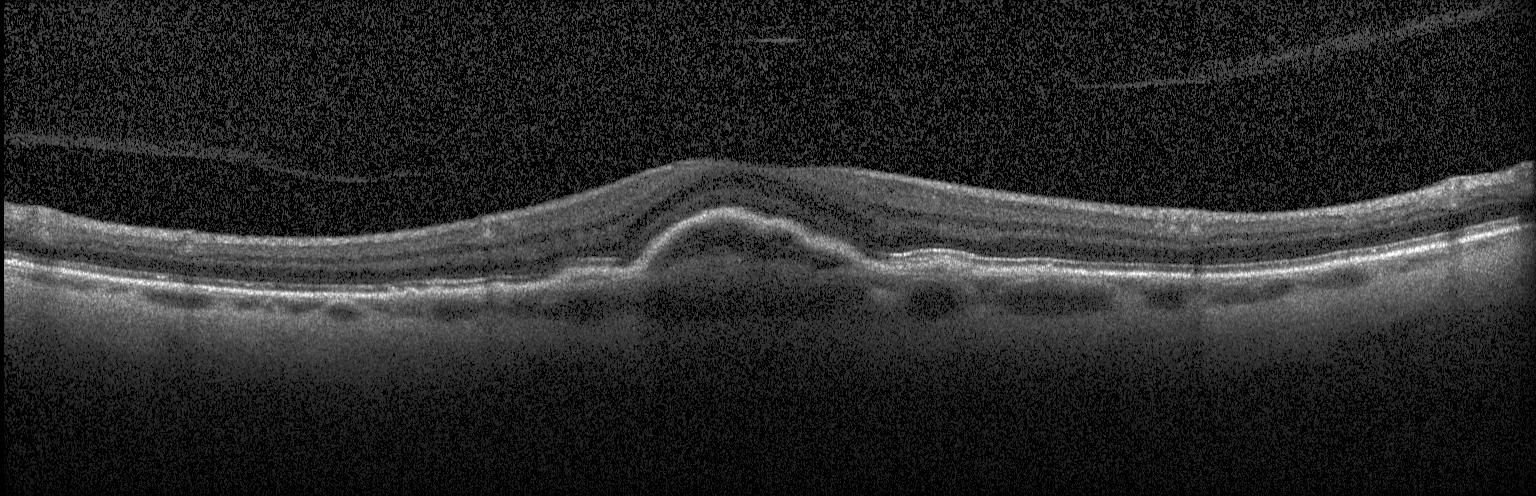

Retinal OCT B-scan · acquired on a Heidelberg Spectralis — Finding: a choroidal neovascular membrane.